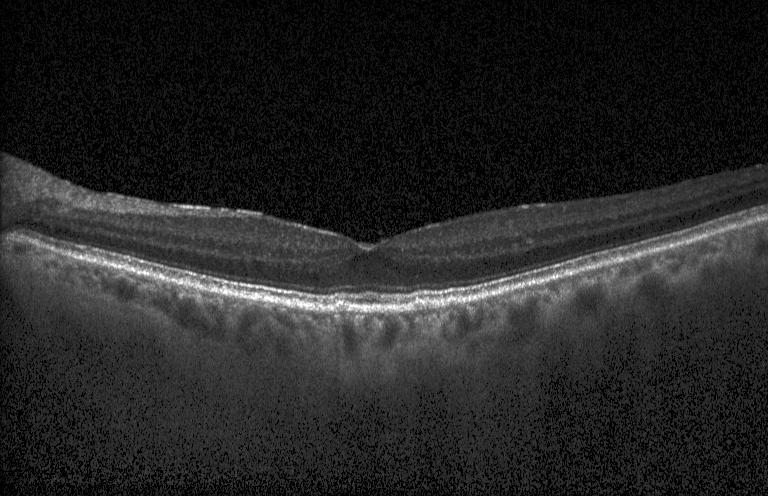 Diagnosis: drusen.